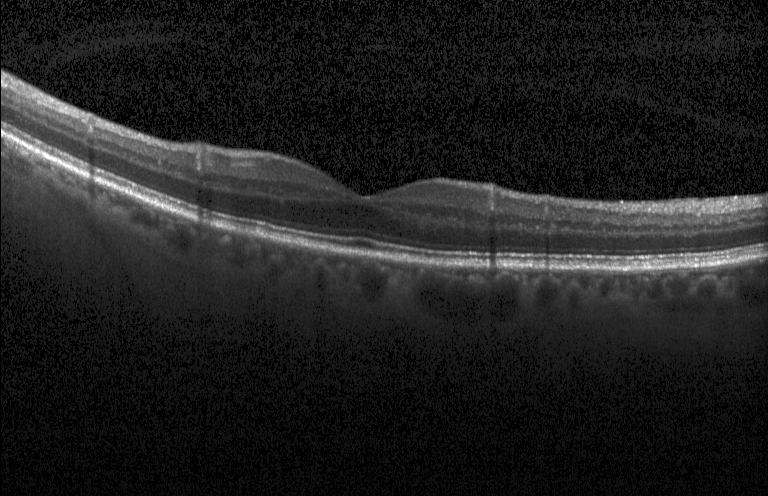
Macular OCT demonstrating no choroidal neovascularization, no diabetic macular edema, and no drusen.